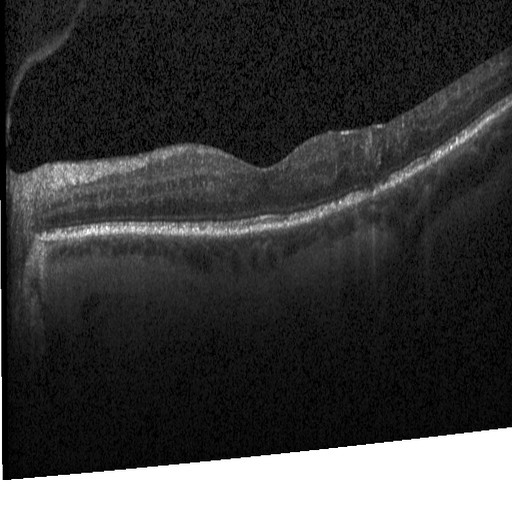

Optical coherence tomography scan. Heidelberg Spectralis OCT system. SD-OCT. Through the macula
Finding: diabetic macular edema.